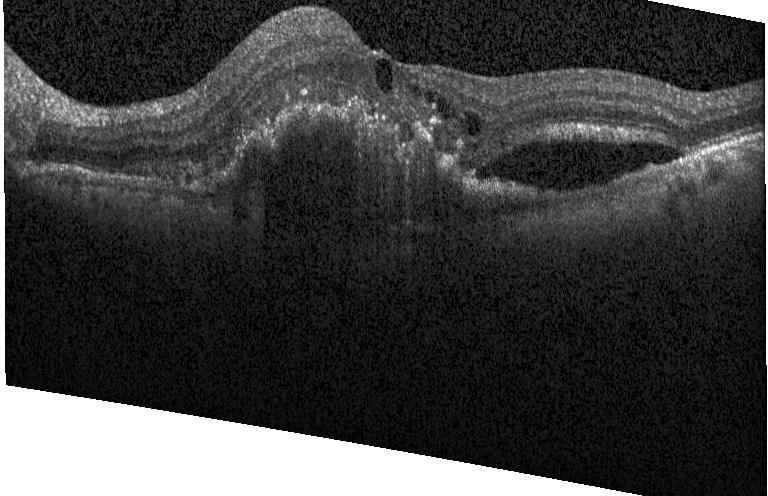 Heidelberg Spectralis OCT system · optical coherence tomography scan
Finding: a choroidal neovascular membrane.